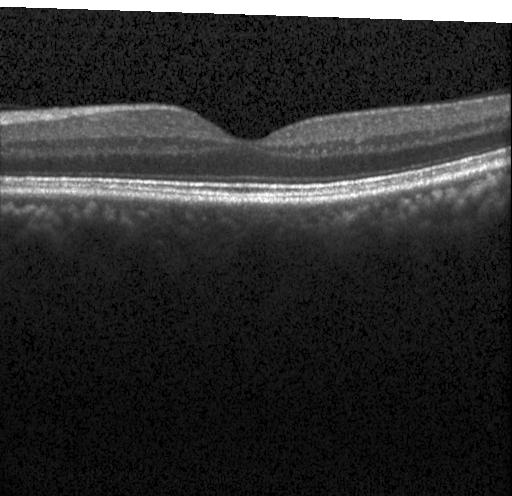 Macular OCT: no choroidal neovascularization, diabetic macular edema, or drusen.